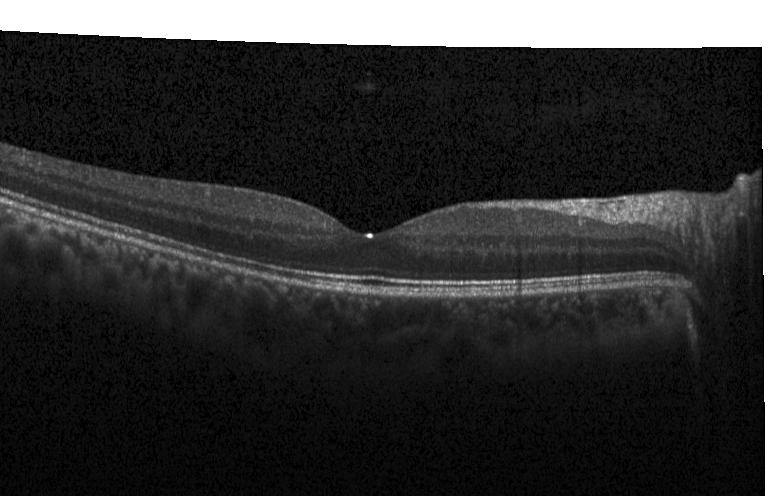 Retinal OCT cross-section · macular scan · Heidelberg Spectralis.
Impression: neither choroidal neovascularization, diabetic macular edema, nor drusen.